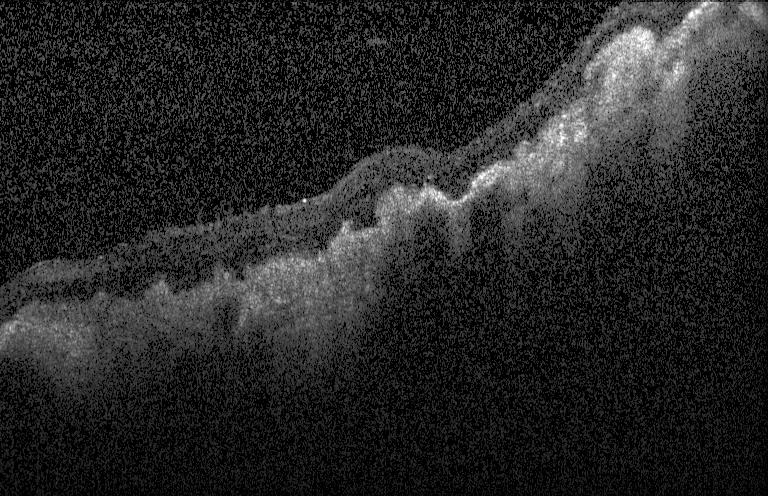

Instrument: Heidelberg Spectralis, optical coherence tomography B-scan.
Assessment: a choroidal neovascular membrane.